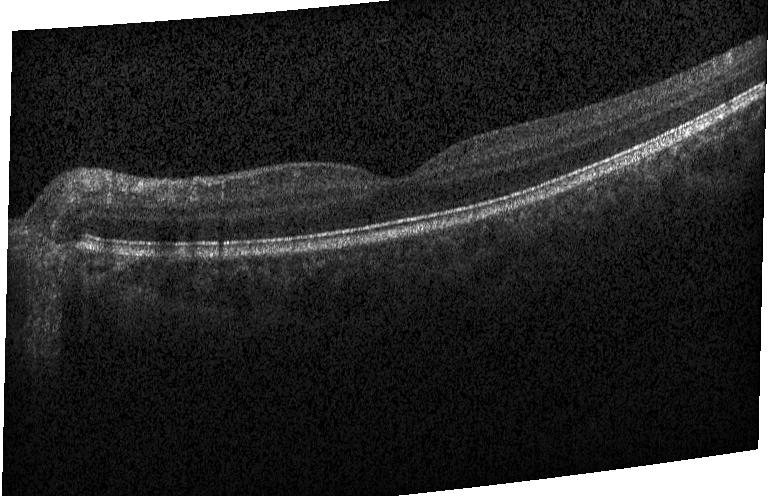

Finding: no choroidal neovascularization, diabetic macular edema, or drusen.